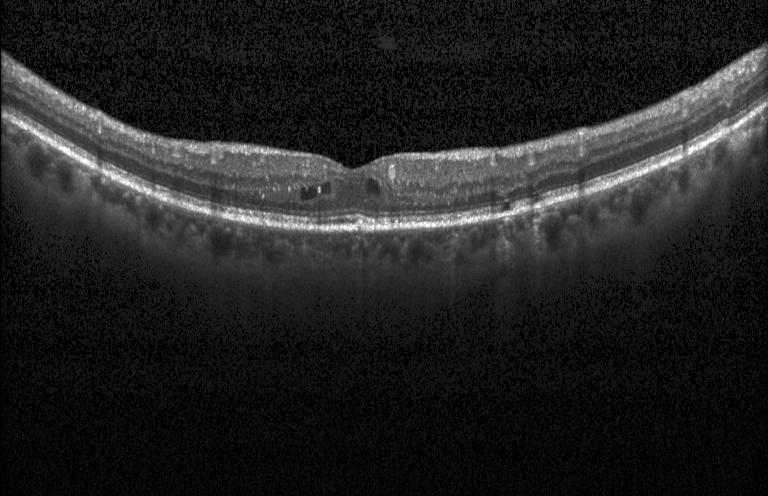
Heidelberg Spectralis. Fovea-centered. Optical coherence tomography B-scan. OCT finding: DME.